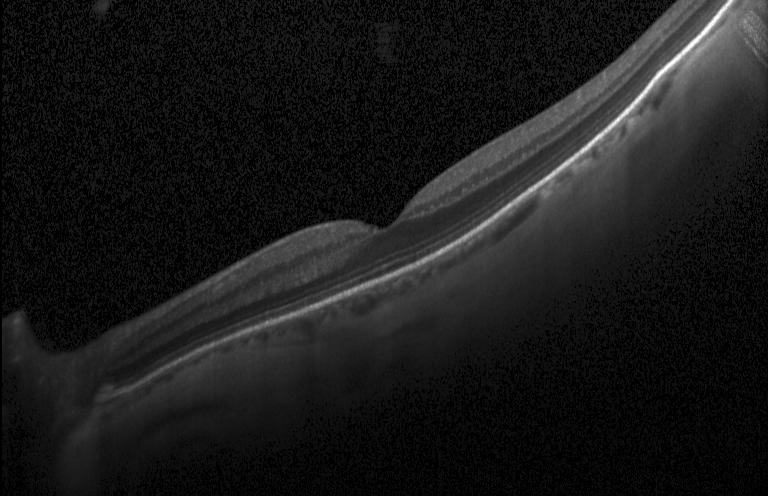 The scan shows no choroidal neovascularization, diabetic macular edema, or drusen.